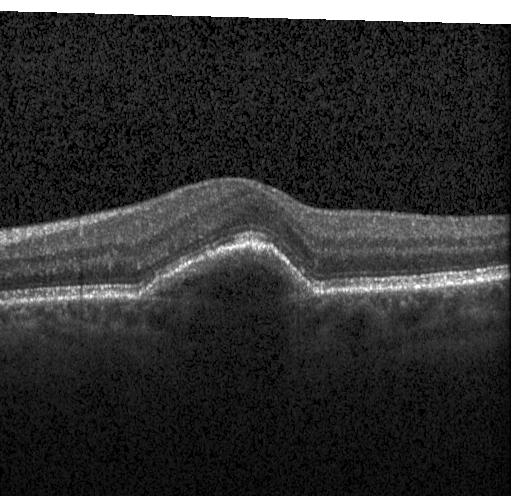

OCT B-scan
Impression: CNV.